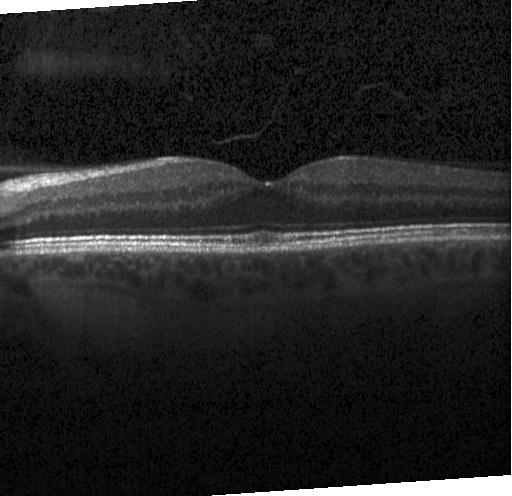 SD-OCT. Through the macula. Heidelberg Spectralis OCT system. Retinal OCT B-scan.
Macular OCT: no CNV, no DME, and no drusen.